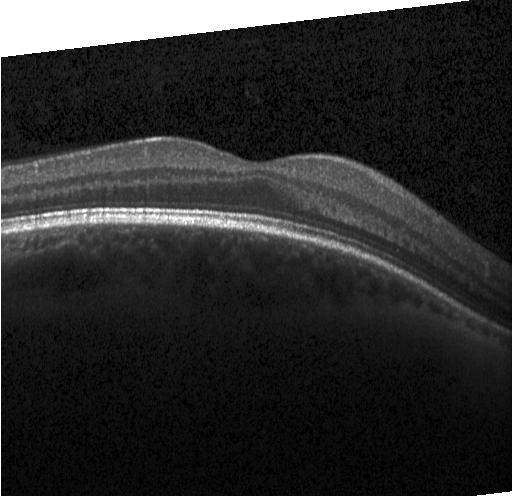
Retinal OCT B-scan · Heidelberg Spectralis OCT system · spectral-domain optical coherence tomography.
OCT finding: no choroidal neovascularization, no diabetic macular edema, and no drusen.